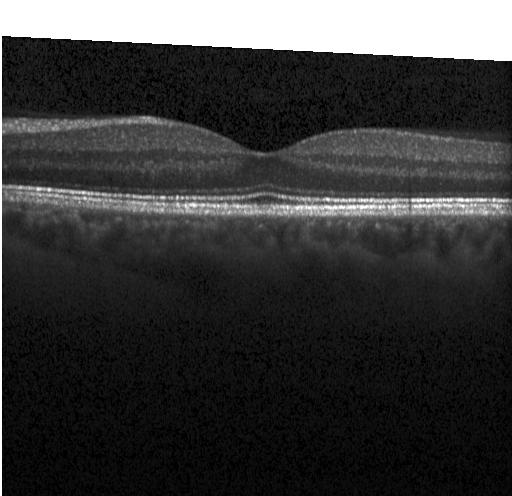
OCT finding: no CNV, DME, or drusen.